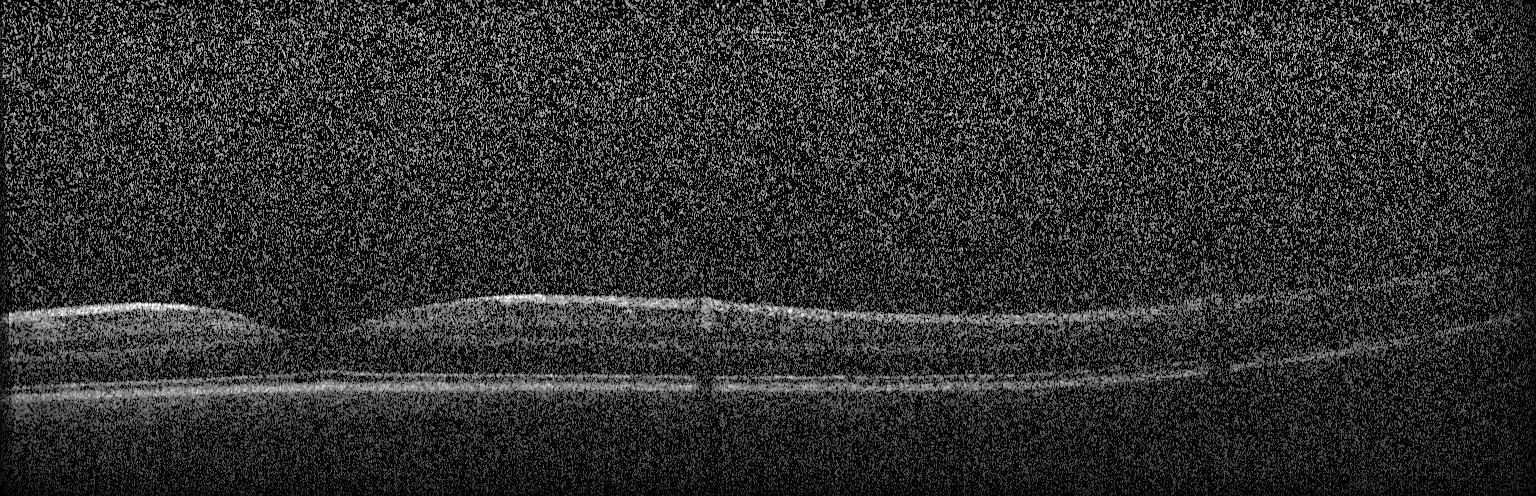 OCT line scan, spectral-domain optical coherence tomography.
Impression: no evidence of choroidal neovascularization, diabetic macular edema, or drusen.